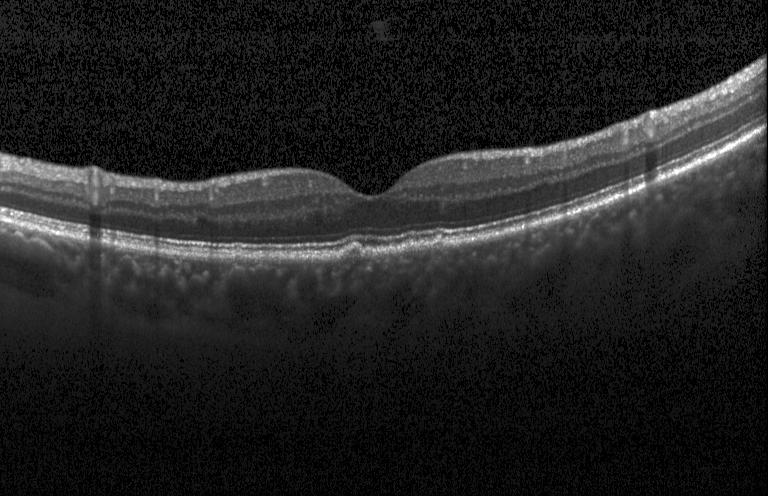

Retinal OCT cross-section · horizontal scan through the fovea · spectral-domain optical coherence tomography · acquired on a Heidelberg Spectralis. OCT finding: sub-RPE drusenoid deposits.